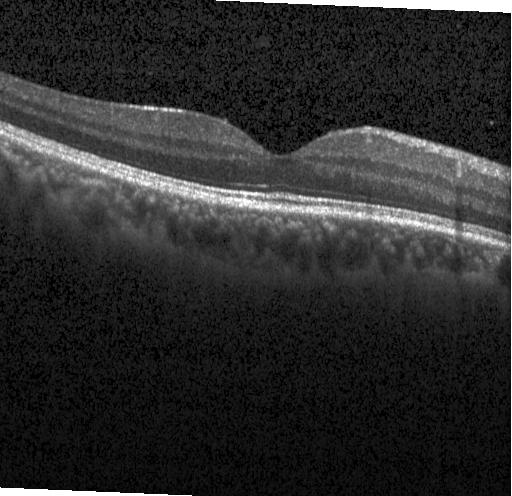

Macular scan, OCT B-scan, SD-OCT, instrument: Heidelberg Spectralis — Finding: no evidence of CNV, DME, or drusen.